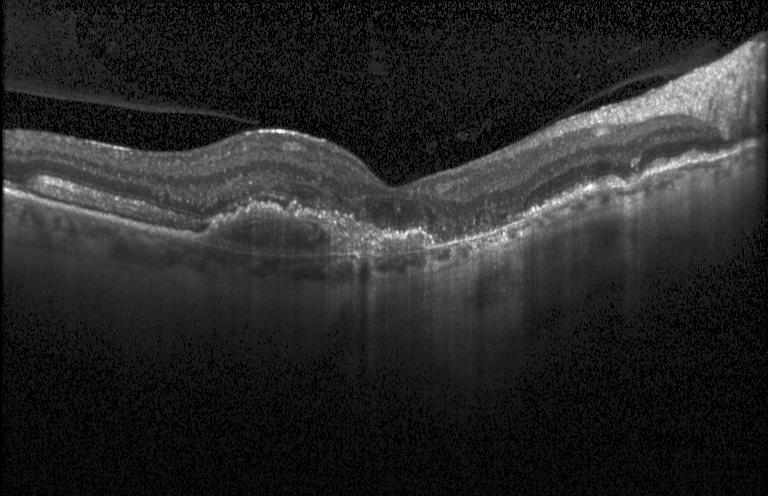
Finding: CNV.